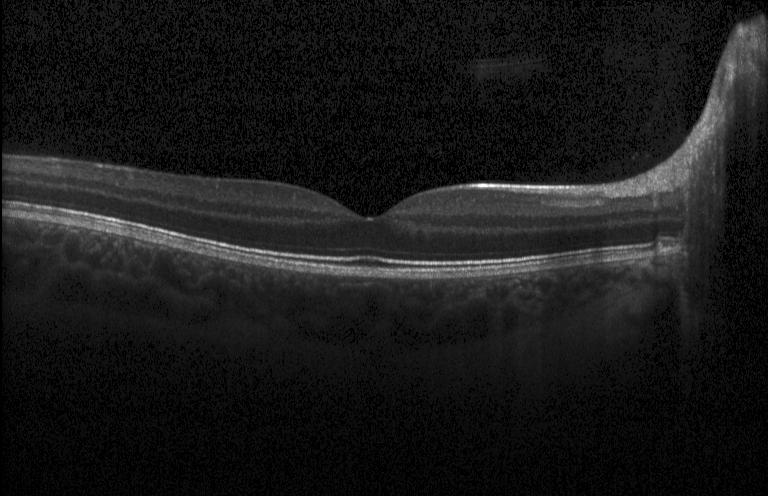 OCT line scan. Horizontal scan through the fovea
Macular OCT: neither choroidal neovascularization, diabetic macular edema, nor drusen.